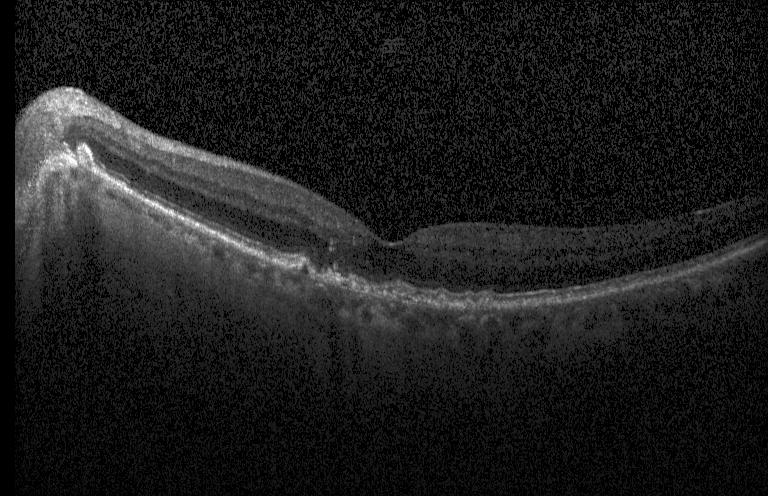
Finding: a choroidal neovascular membrane.